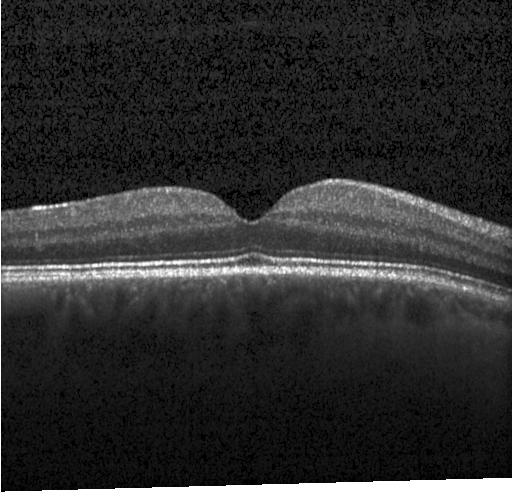 Assessment: neither CNV, DME, nor drusen.